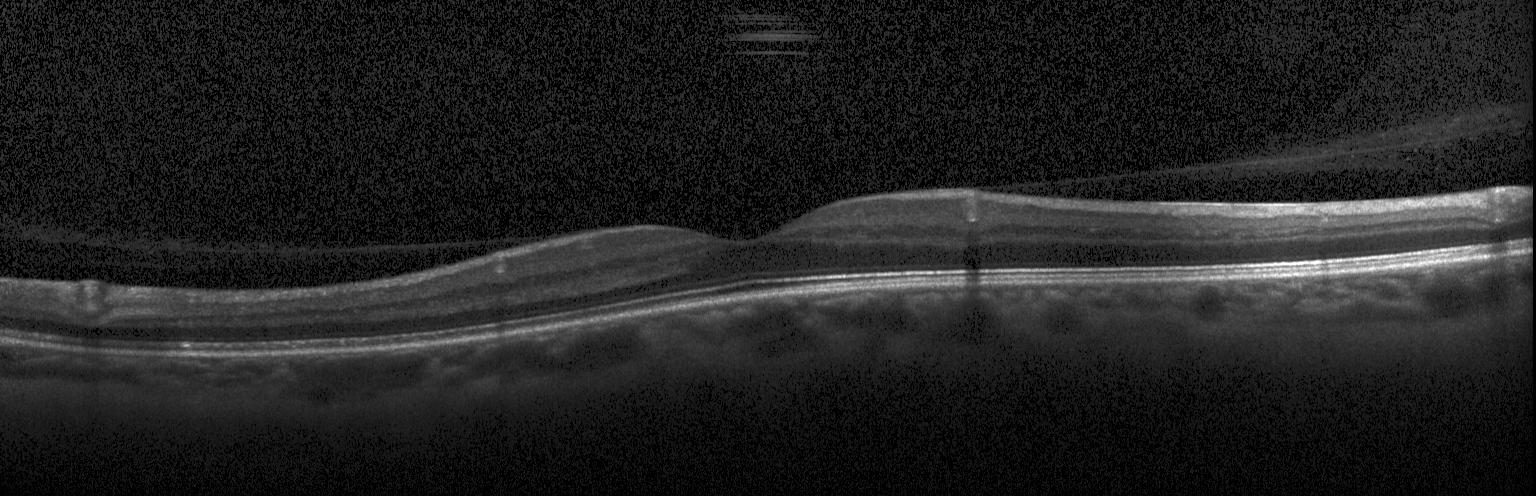
Macular scan · retinal OCT cross-section. Finding: no choroidal neovascularization, no diabetic macular edema, and no drusen.